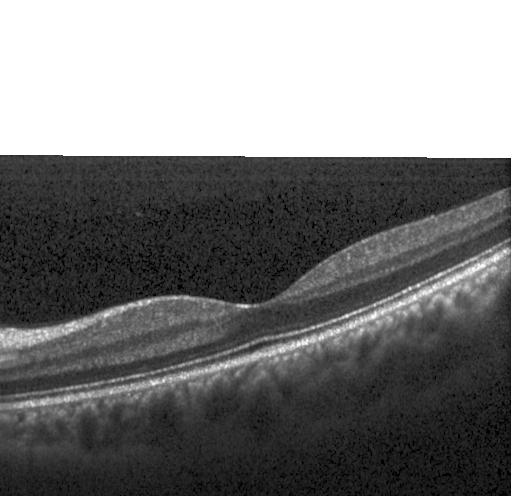
Retinal OCT B-scan · through the macula · instrument: Heidelberg Spectralis · spectral-domain OCT. Macular OCT: neither choroidal neovascularization, diabetic macular edema, nor drusen.